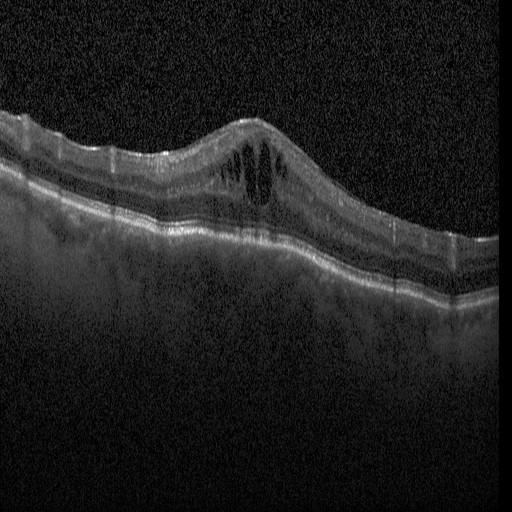

OCT finding: DME.